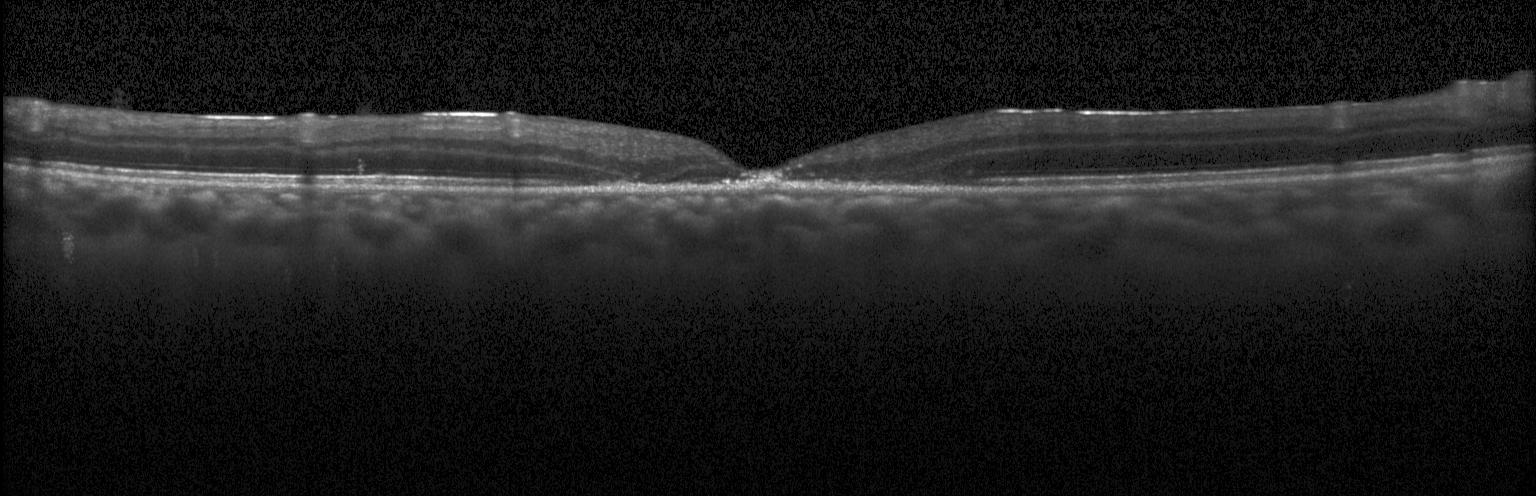
Heidelberg Spectralis; OCT B-scan. Diagnosis: neither CNV, DME, nor drusen.